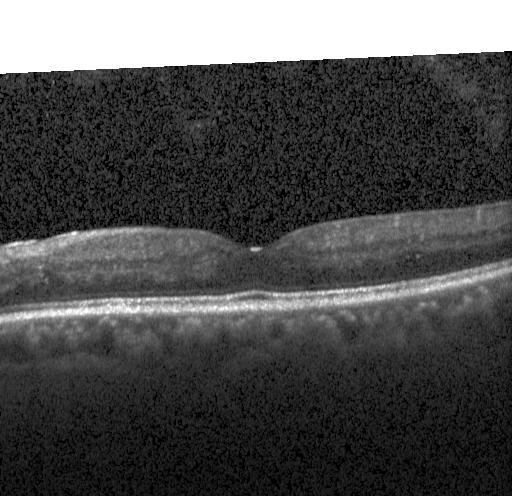
OCT scan showing no evidence of CNV, DME, or drusen.